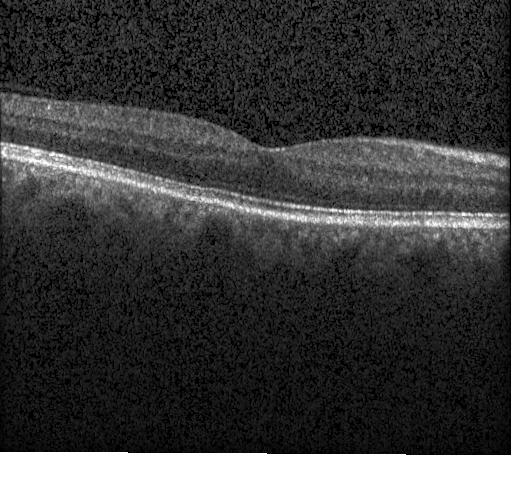

Optical coherence tomography B-scan — Diagnosis: no choroidal neovascularization, diabetic macular edema, or drusen.